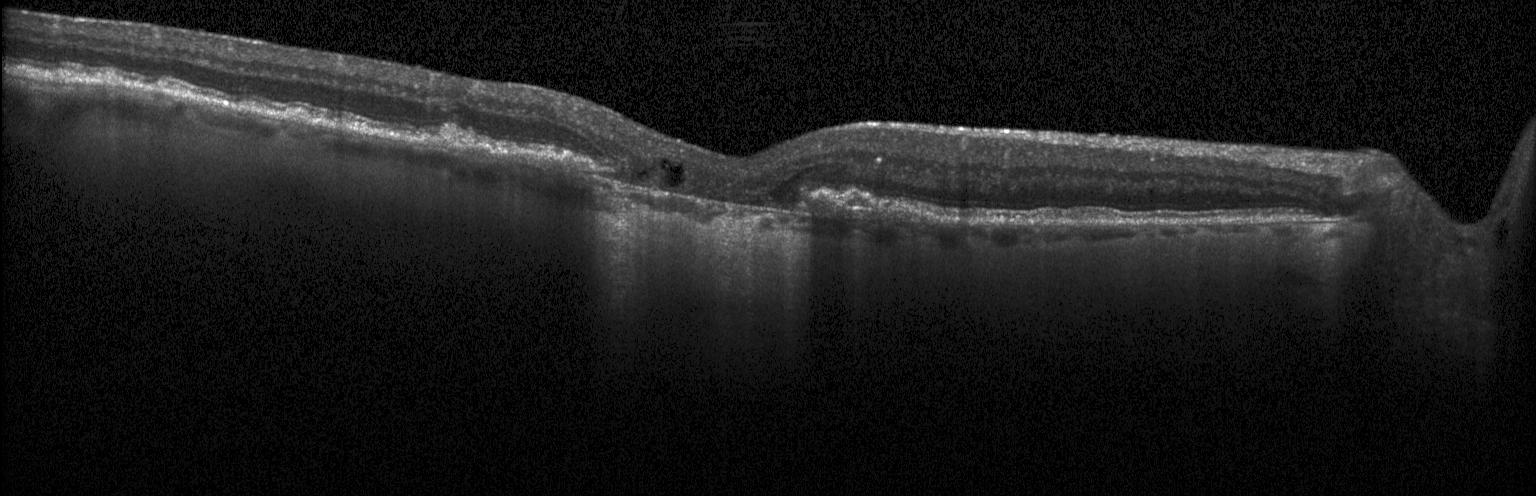
Optical coherence tomography scan. Assessment: choroidal neovascularization.